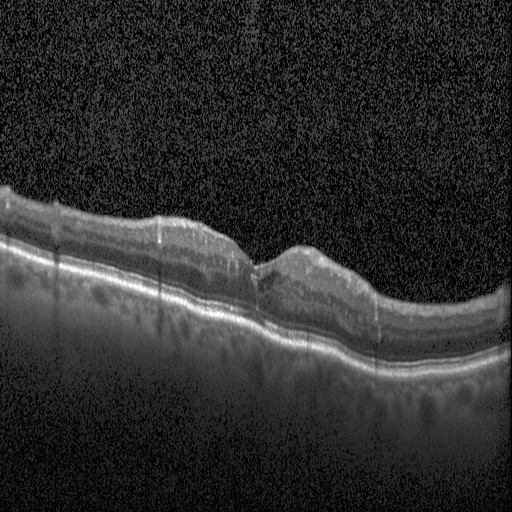
Dx: diabetic macular edema (DME).